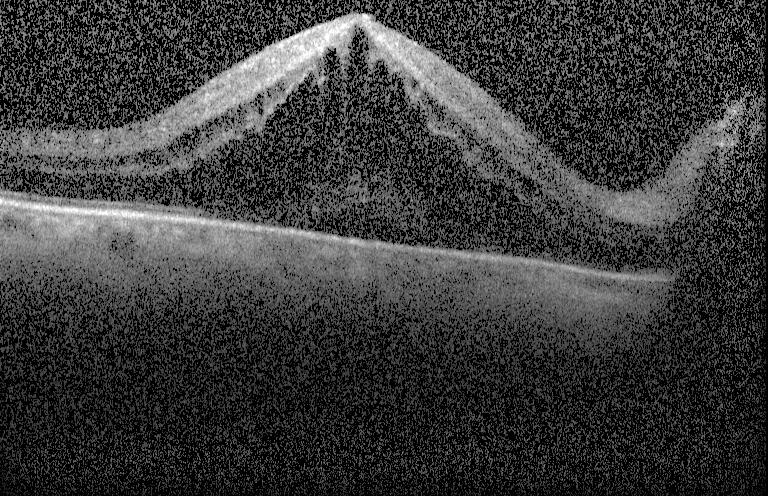
Impression: diabetic macular edema (DME).